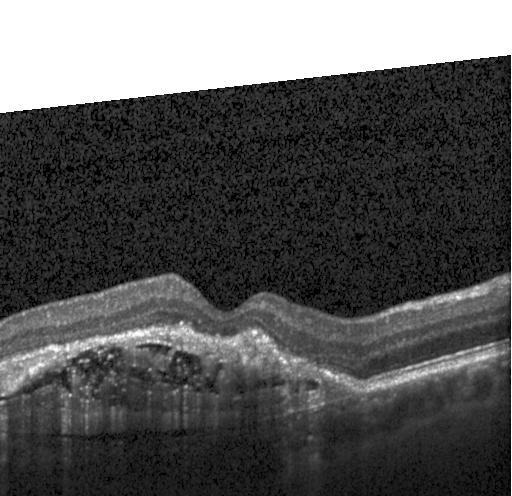 Macular scan · optical coherence tomography scan. Diagnosis: CNV.